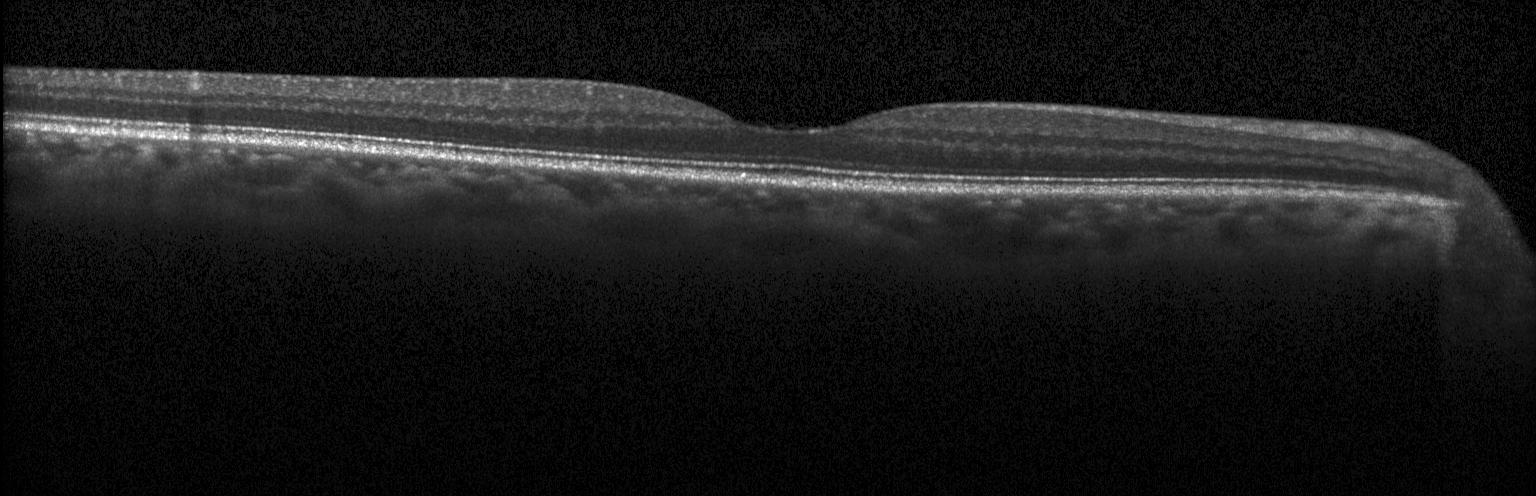

Impression: no evidence of choroidal neovascularization, diabetic macular edema, or drusen.